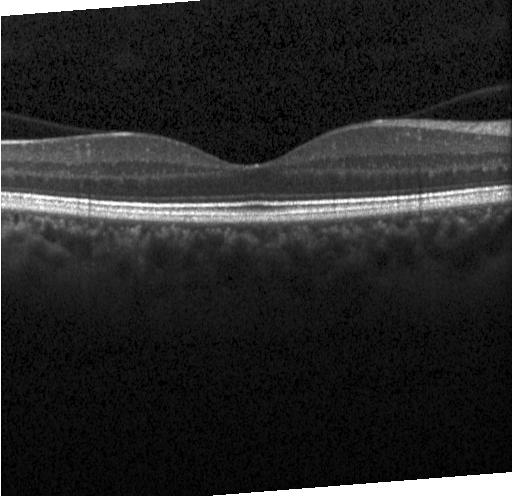
Retinal OCT B-scan
Assessment: no CNV, DME, or drusen.